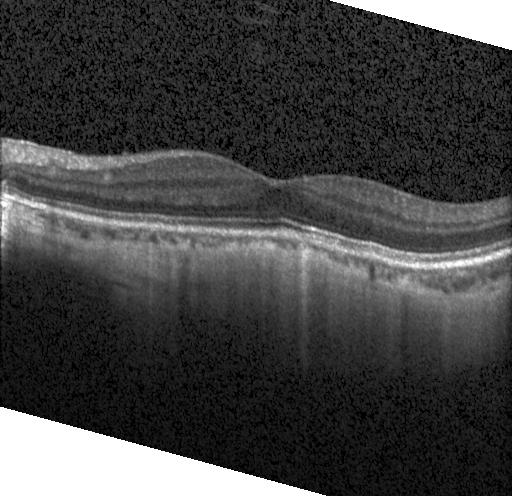

Impression: no choroidal neovascularization, diabetic macular edema, or drusen.